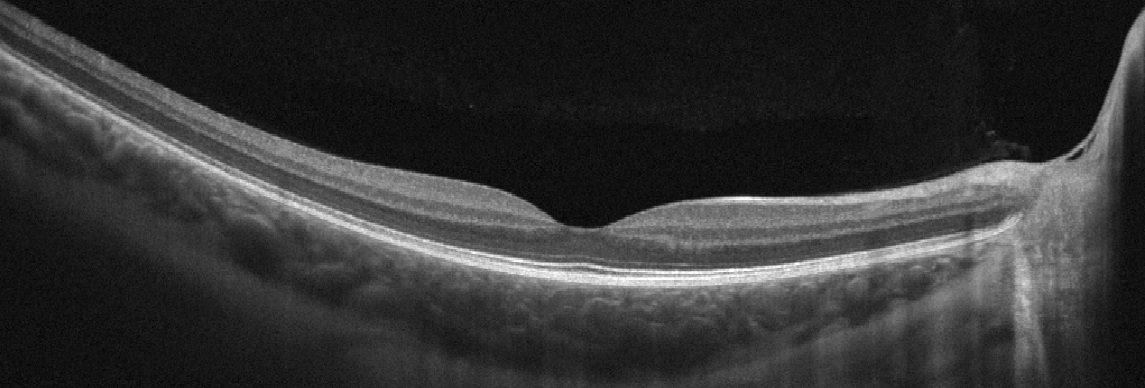

Instrument: Optovue Avanti RTVue XR. Retinal OCT cross-section. Macular scan — The scan shows no evidence of AMD, DME, ERM, RAO, RVO, or VID.